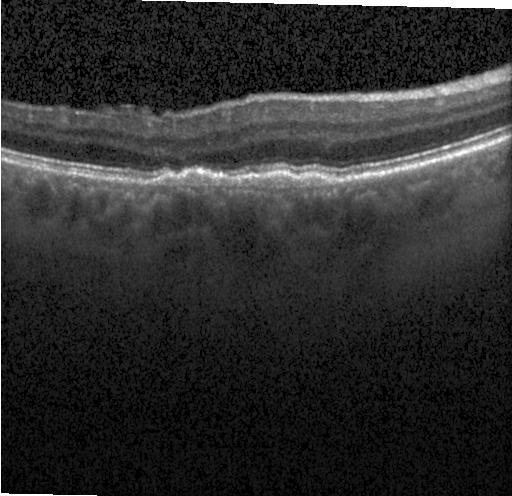

Diagnosis: choroidal neovascularization (CNV).